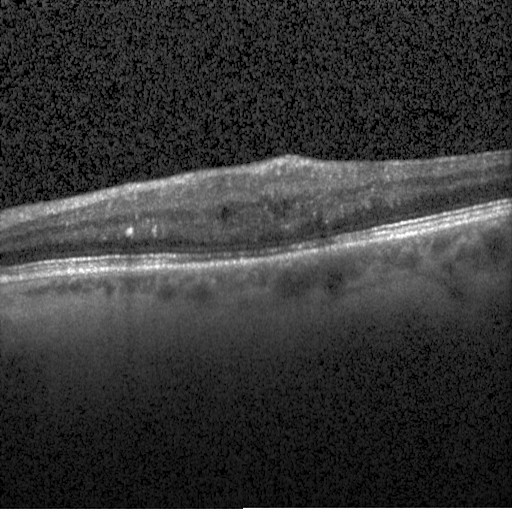 Assessment: diabetic macular edema (DME).